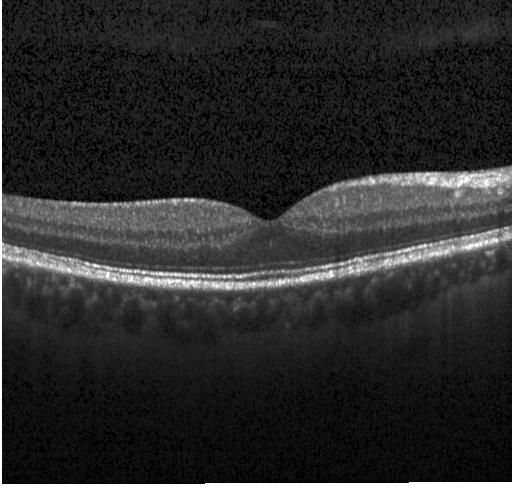

Fovea-centered; retinal OCT cross-section
Finding: no evidence of choroidal neovascularization, diabetic macular edema, or drusen.